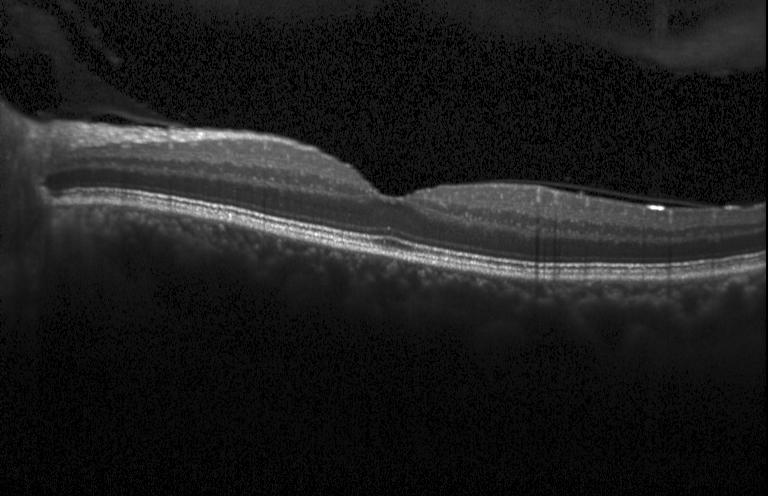

OCT finding: no choroidal neovascularization, no diabetic macular edema, and no drusen.